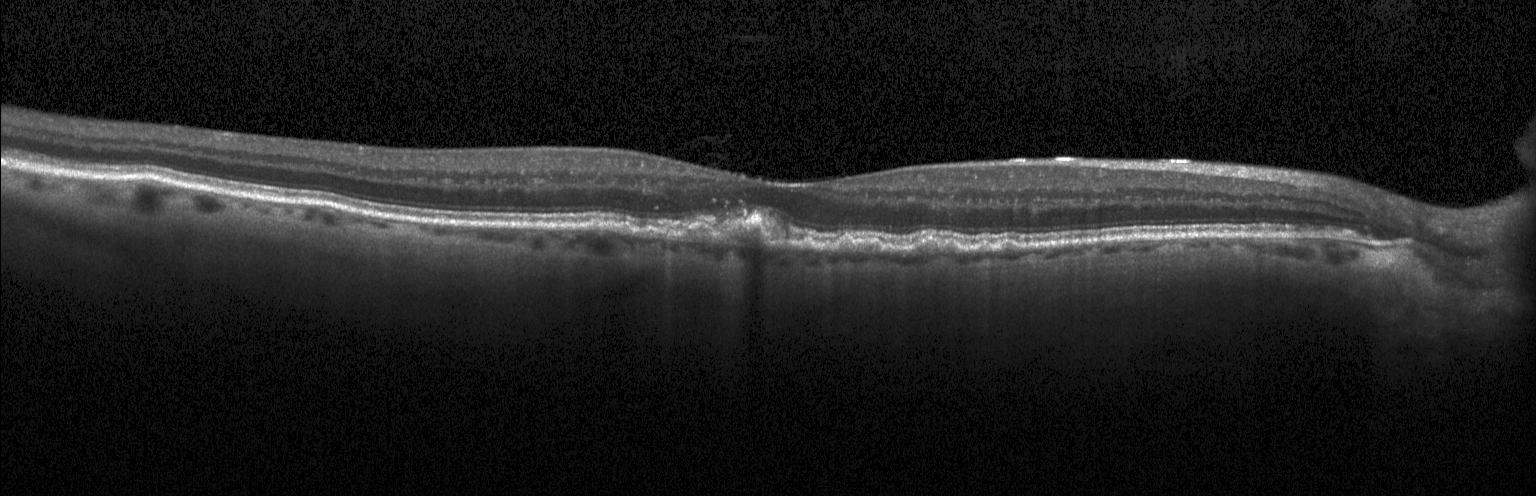 Spectral-domain optical coherence tomography · fovea-centered · retinal OCT cross-section — This B-scan demonstrates sub-RPE drusenoid deposits.